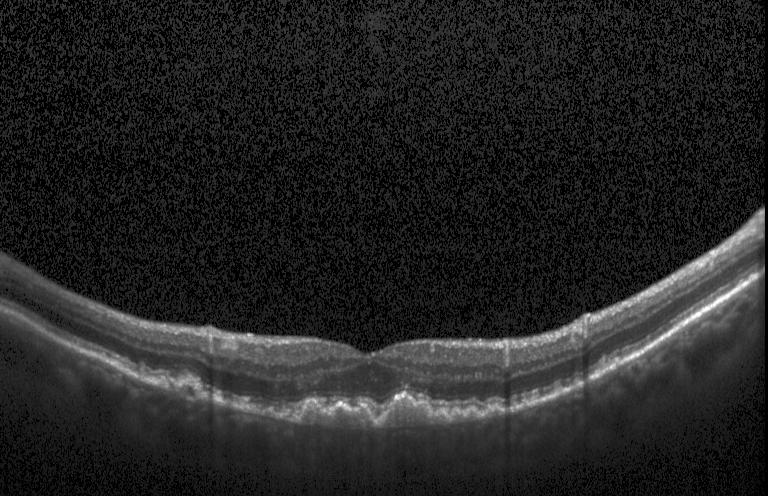

OCT scan showing sub-RPE drusenoid deposits.